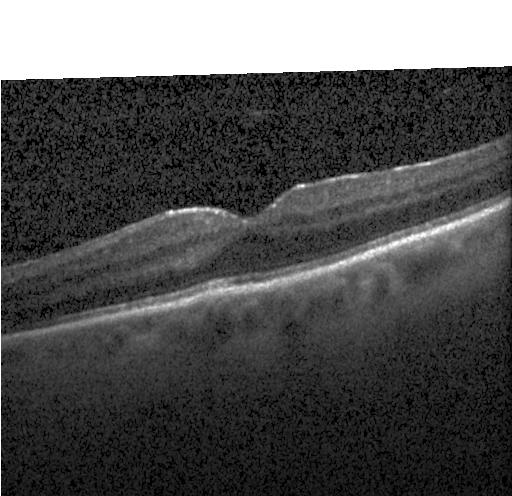
Optical coherence tomography B-scan. Spectral-domain optical coherence tomography. Instrument: Heidelberg Spectralis — OCT finding: neither CNV, DME, nor drusen.